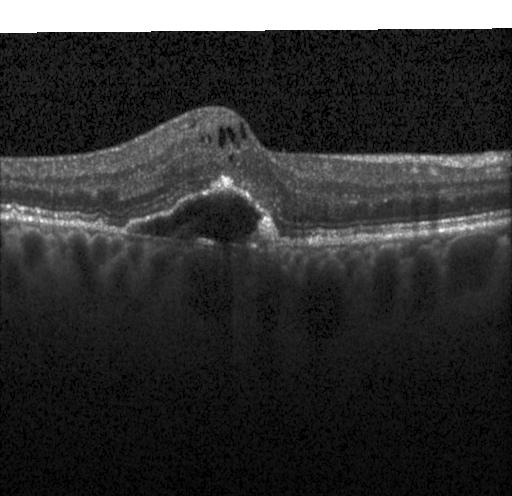

Optical coherence tomography B-scan. SD-OCT
Choroidal neovascularization (CNV).